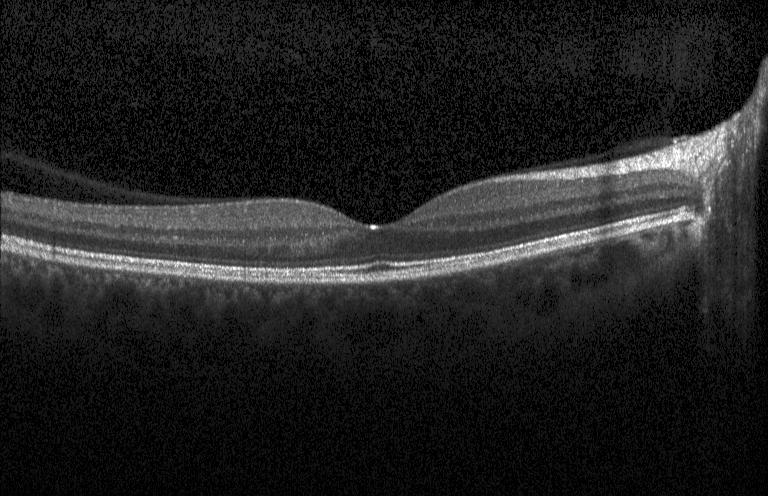 Optical coherence tomography scan · macular scan · spectral-domain optical coherence tomography · acquired on a Heidelberg Spectralis.
The scan shows no evidence of choroidal neovascularization, diabetic macular edema, or drusen.